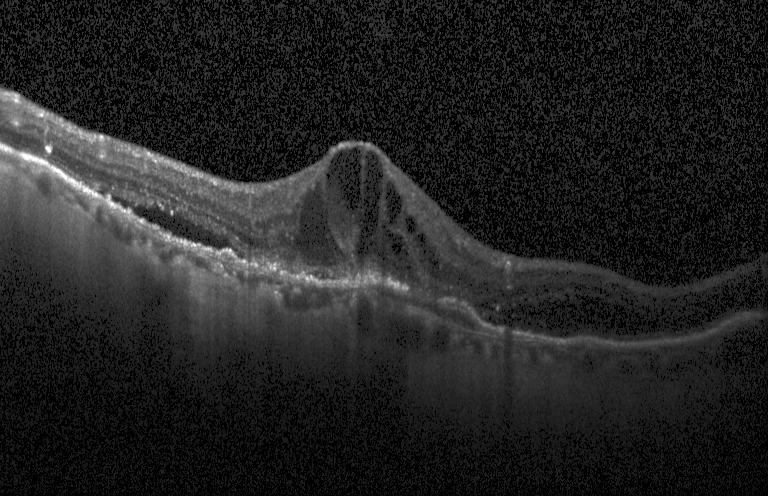 Diagnosis: choroidal neovascularization (CNV).